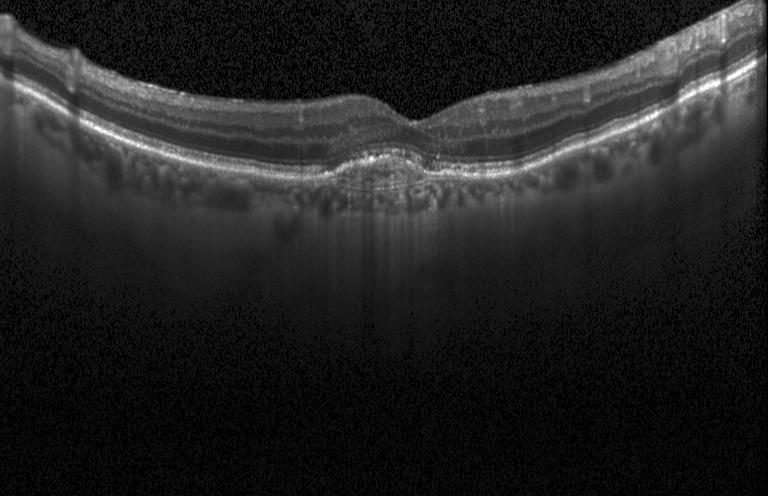

SD-OCT · retinal OCT cross-section
Impression: a choroidal neovascular membrane.